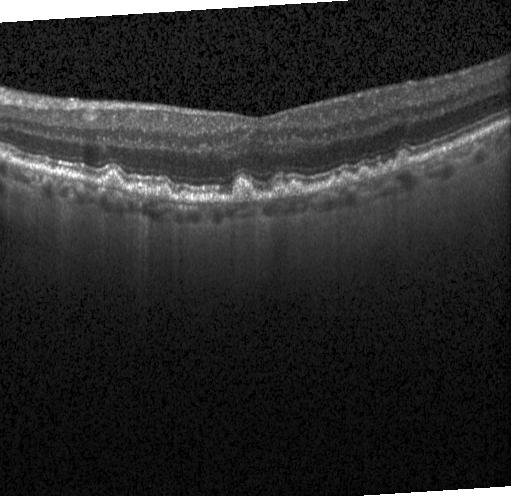
Retinal OCT B-scan
Dx: sub-RPE drusenoid deposits.